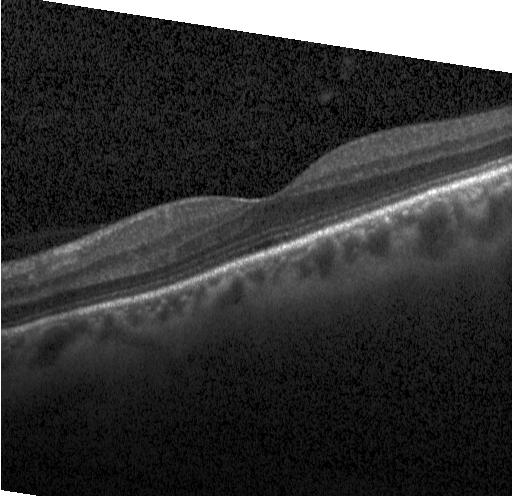 Assessment: neither choroidal neovascularization, diabetic macular edema, nor drusen.